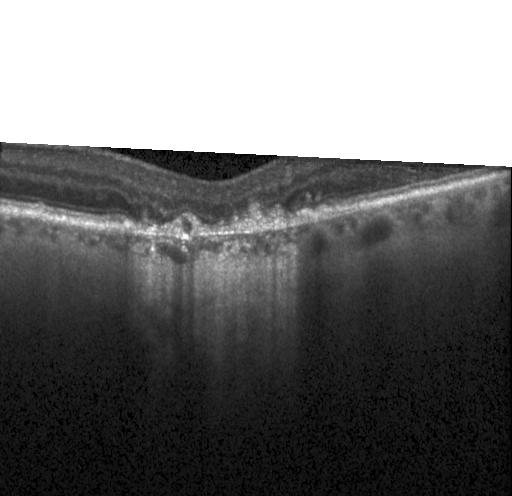
The scan shows a choroidal neovascular membrane.